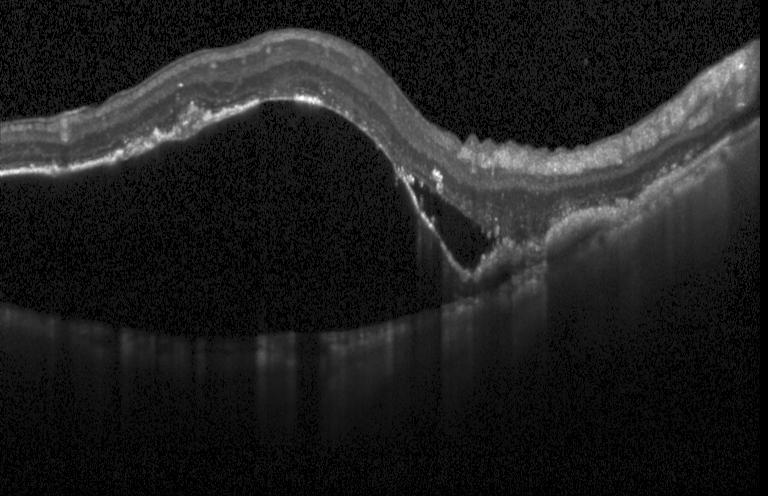
Impression: a choroidal neovascular membrane.